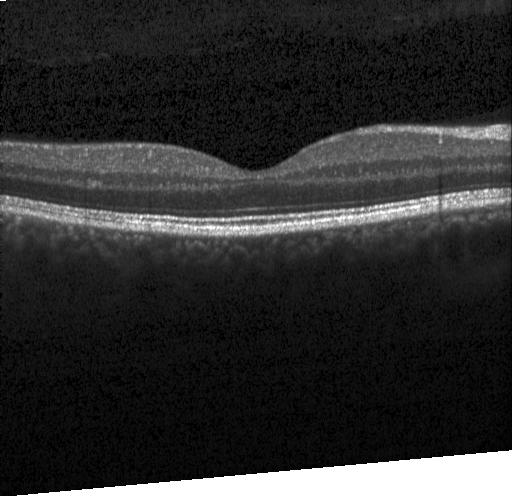
Through the macula; Heidelberg Spectralis OCT system; SD-OCT; OCT B-scan
Impression: no choroidal neovascularization, diabetic macular edema, or drusen.